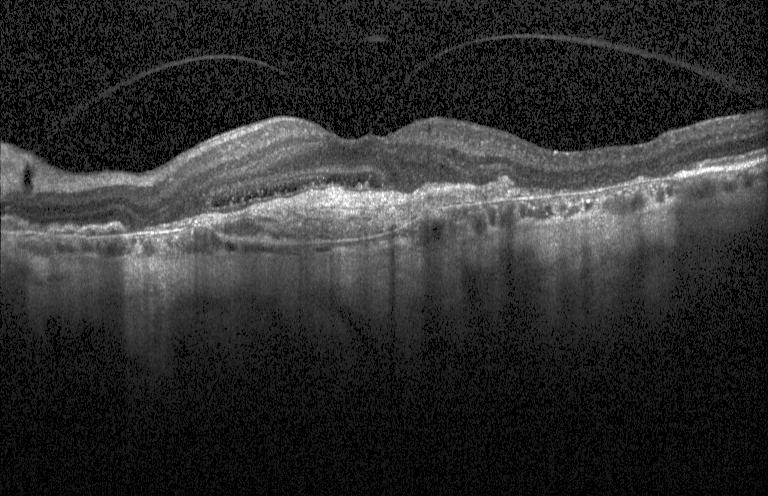
Spectral-domain OCT B-scan: choroidal neovascularization (CNV).